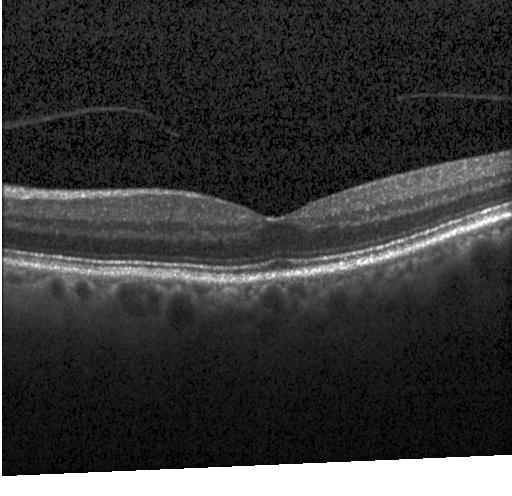 OCT finding: neither CNV, DME, nor drusen.